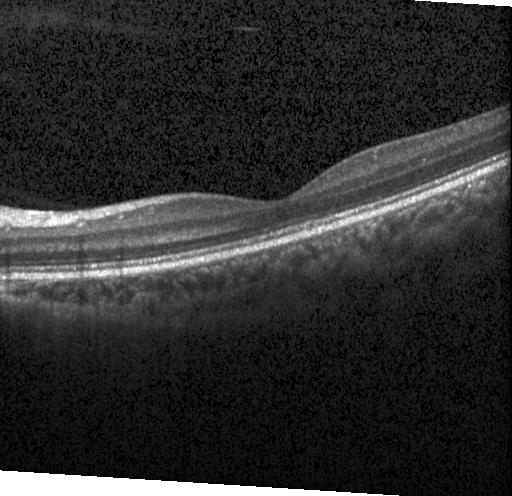
Heidelberg Spectralis; retinal OCT cross-section.
Finding: no choroidal neovascularization, no diabetic macular edema, and no drusen.